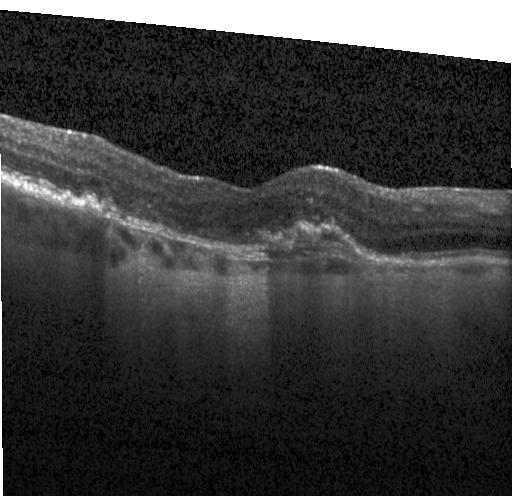
Spectral-domain OCT, acquired on a Heidelberg Spectralis, fovea-centered, optical coherence tomography scan. Impression: a choroidal neovascular membrane.